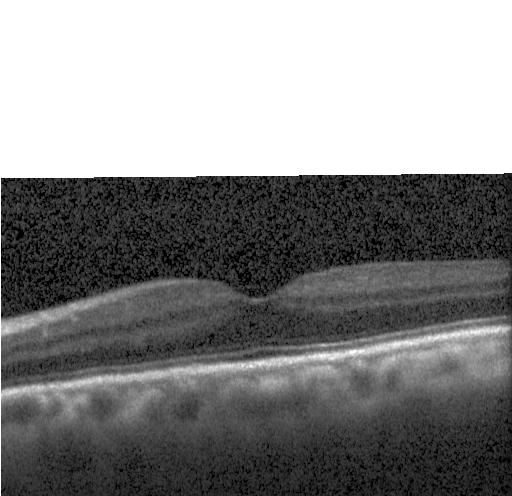

Instrument: Heidelberg Spectralis. SD-OCT. OCT line scan. Macular scan.
Impression: no choroidal neovascularization, no diabetic macular edema, and no drusen.